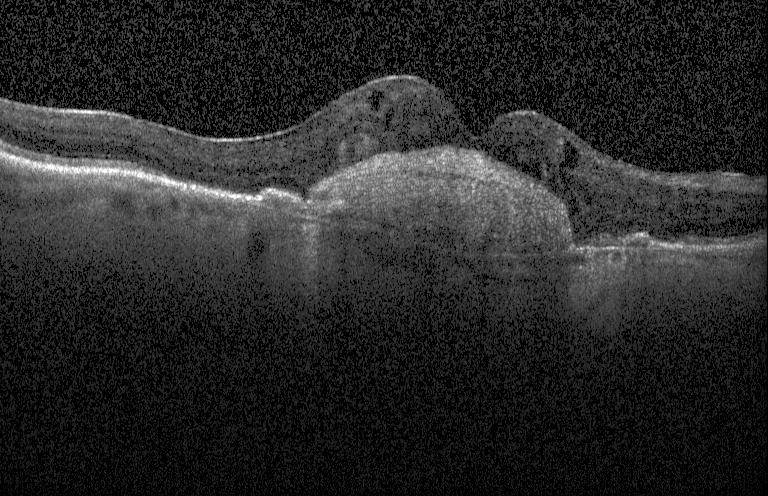 Macular OCT: choroidal neovascularization.